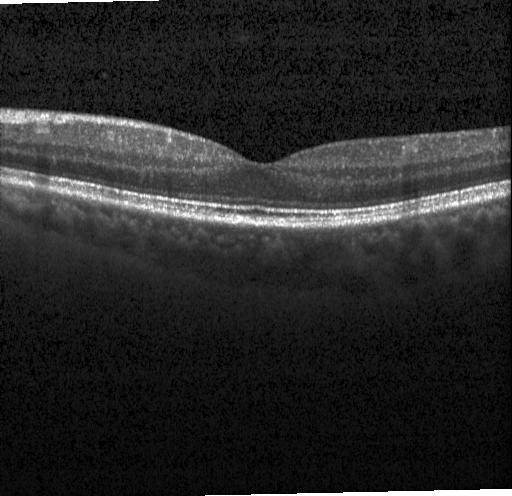
Macular scan, OCT B-scan. Finding: no choroidal neovascularization, diabetic macular edema, or drusen.